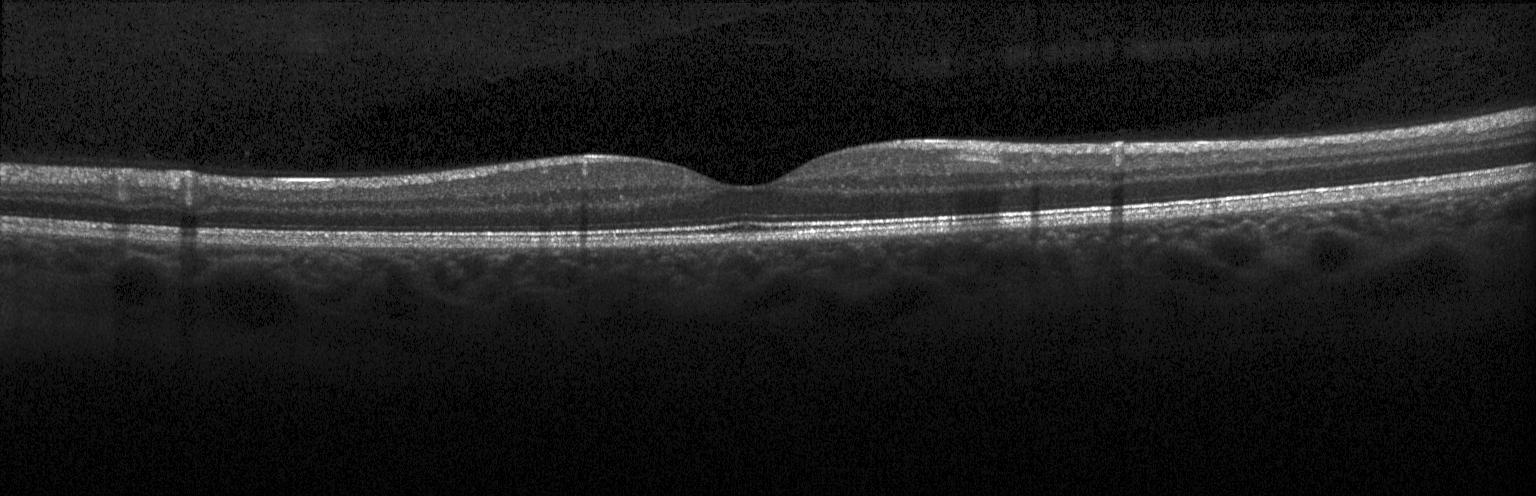

OCT B-scan showing neither choroidal neovascularization, diabetic macular edema, nor drusen.